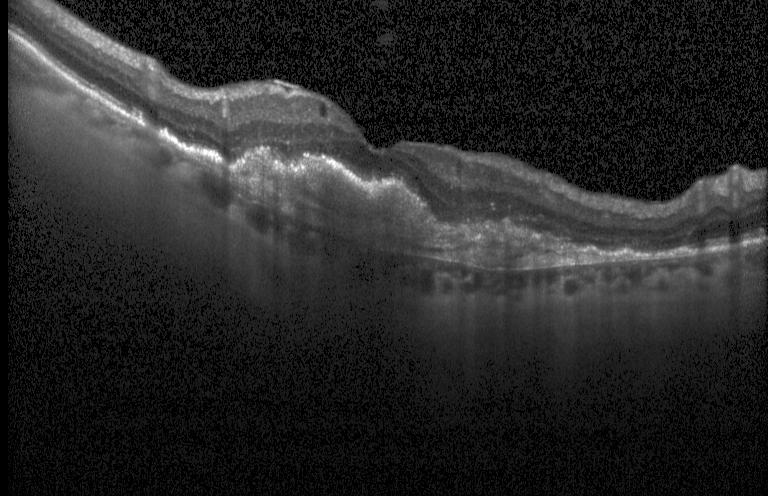
Optical coherence tomography scan
Dx: choroidal neovascularization (CNV).